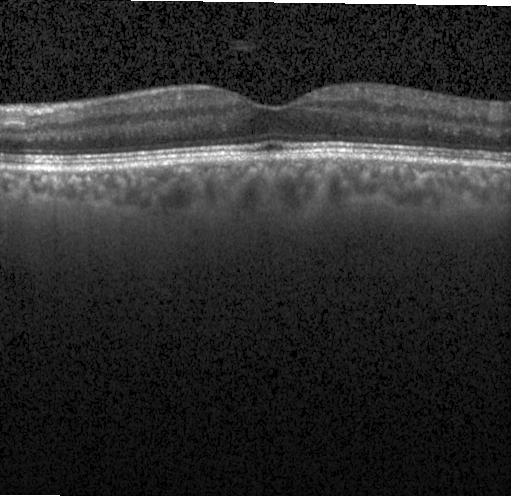 Retinal OCT B-scan — Impression: no evidence of CNV, DME, or drusen.